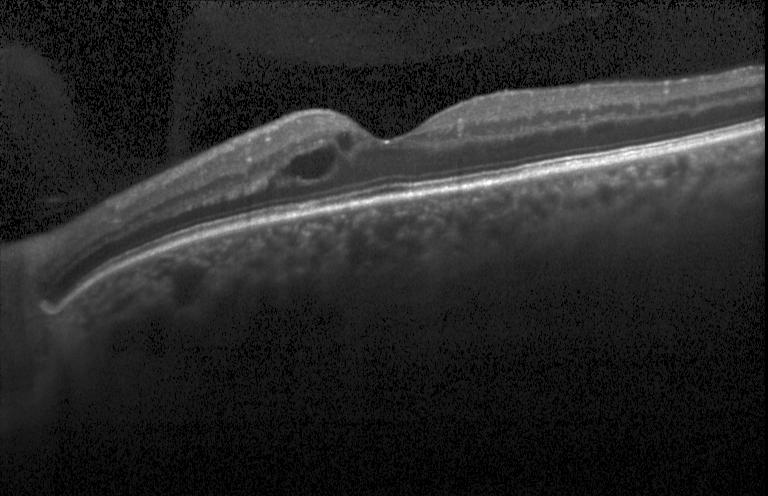
Finding: diabetic macular edema (DME).